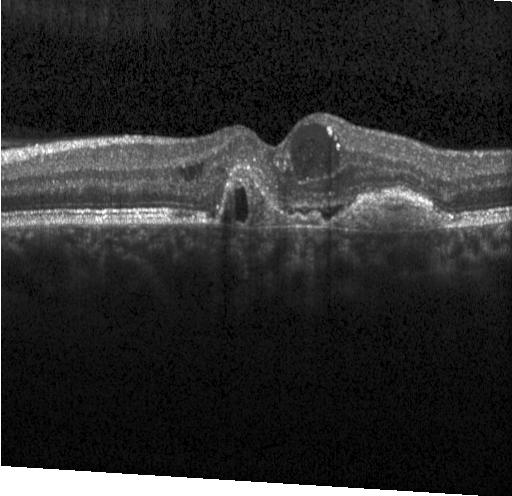 Acquired on a Heidelberg Spectralis. Spectral-domain OCT. OCT line scan — A choroidal neovascular membrane.